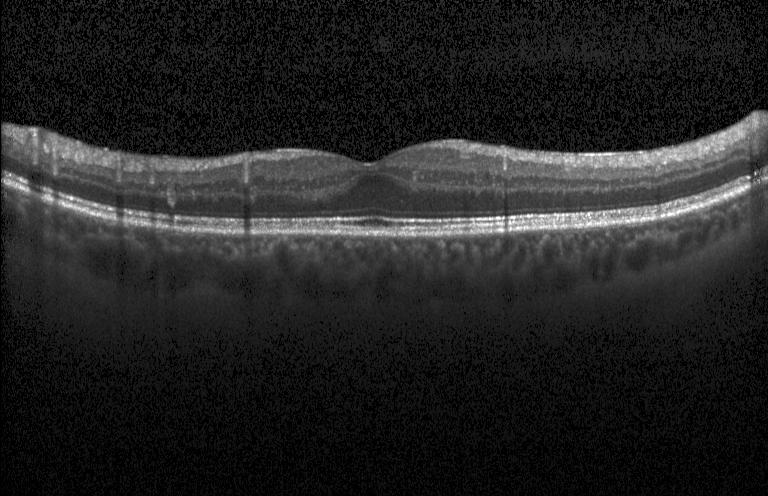

Retinal OCT cross-section showing neither CNV, DME, nor drusen.